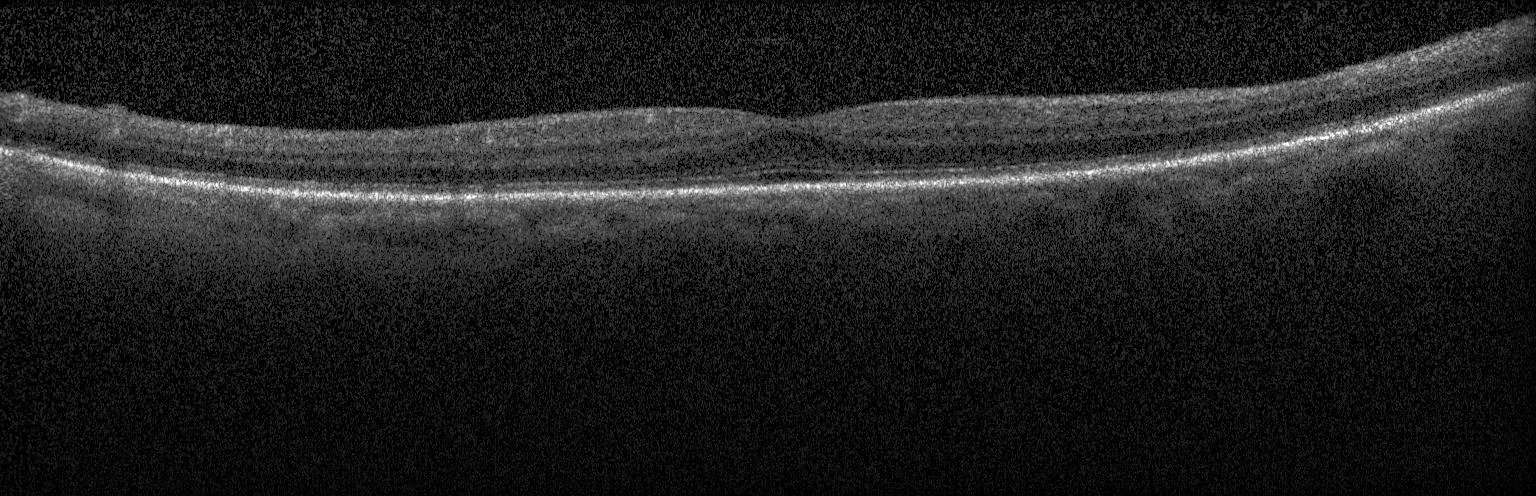 Retinal OCT B-scan.
No evidence of choroidal neovascularization, diabetic macular edema, or drusen.